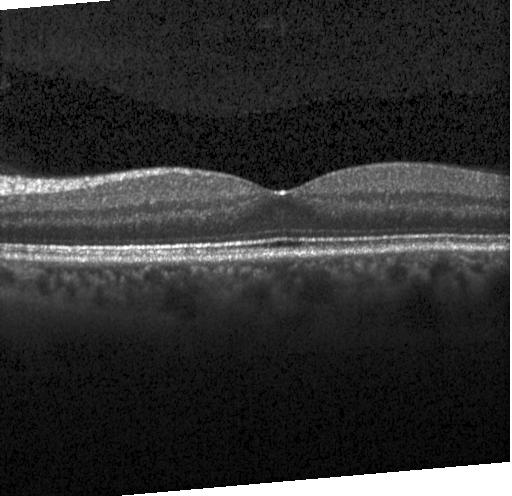 Retinal OCT cross-section · SD-OCT
Macular OCT: no evidence of choroidal neovascularization, diabetic macular edema, or drusen.